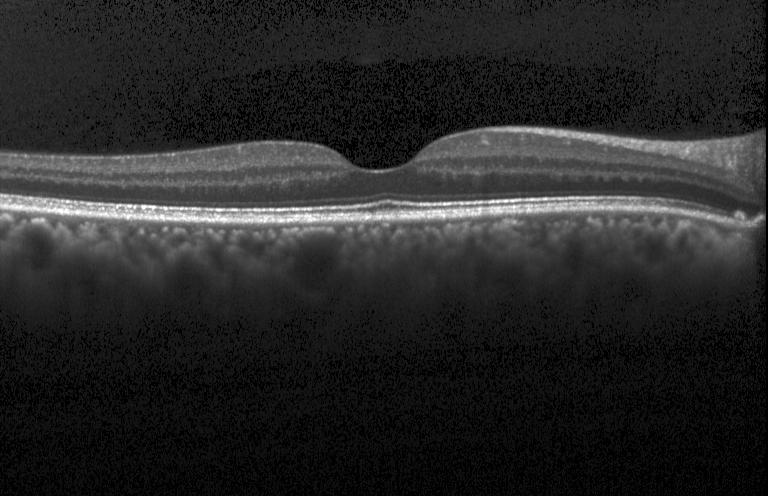 Heidelberg Spectralis OCT system, retinal OCT cross-section, SD-OCT. Diagnosis: no evidence of choroidal neovascularization, diabetic macular edema, or drusen.